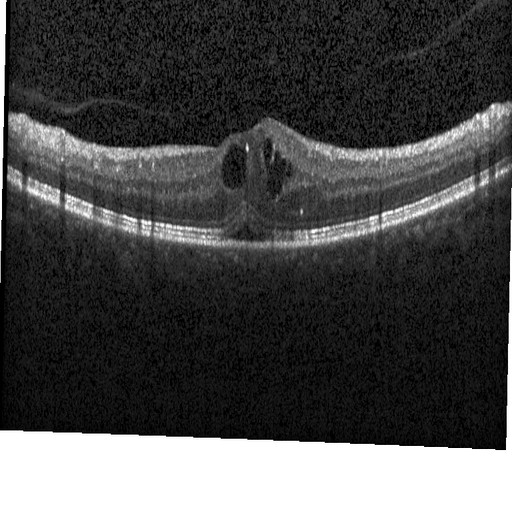 OCT B-scan showing diabetic macular edema.